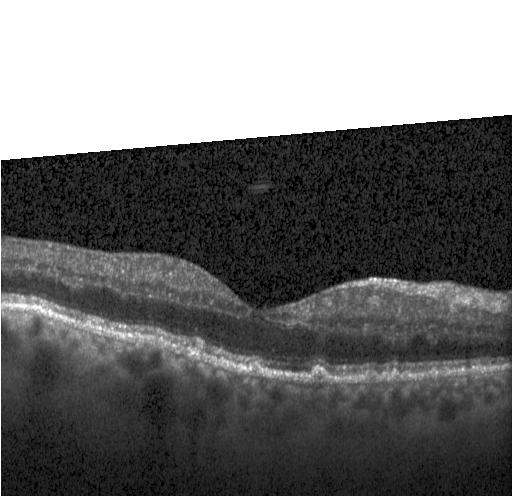

Spectral-domain OCT B-scan: drusen.